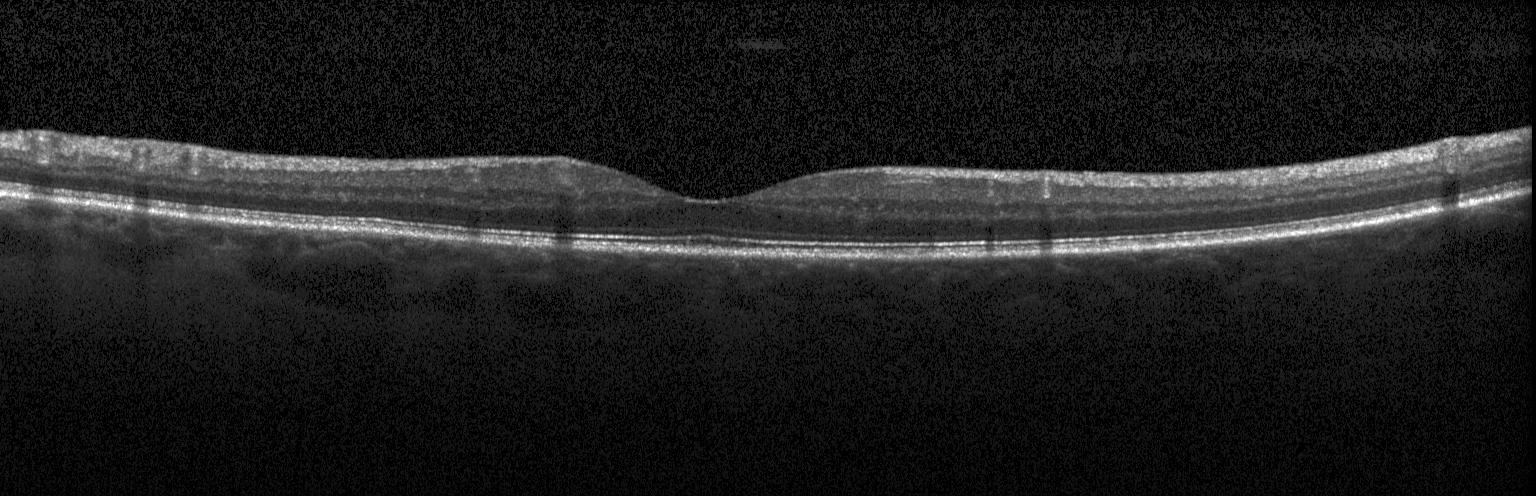 Retinal OCT B-scan; Heidelberg Spectralis OCT system; spectral-domain OCT.
Impression: no choroidal neovascularization, no diabetic macular edema, and no drusen.